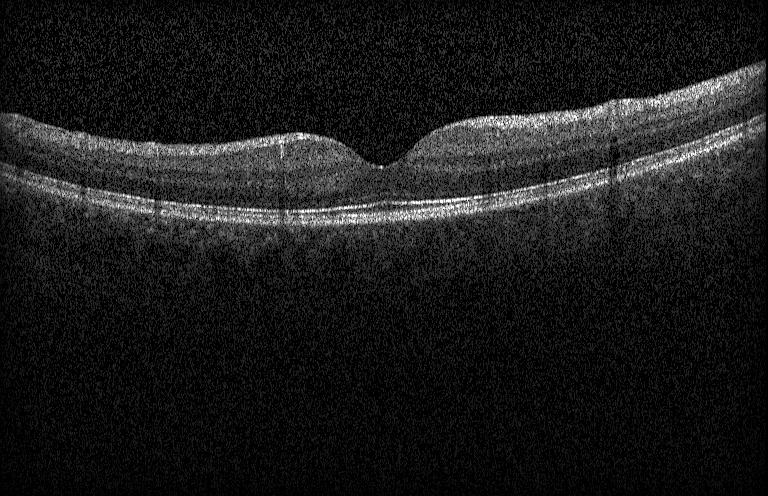 Optical coherence tomography B-scan — Impression: no choroidal neovascularization, diabetic macular edema, or drusen.